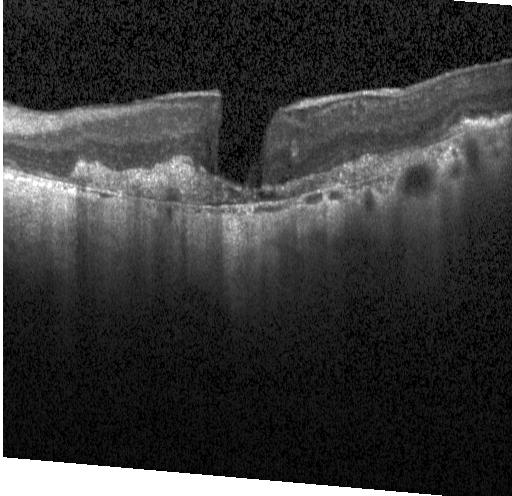 Spectral-domain OCT. Acquired on a Heidelberg Spectralis. Optical coherence tomography scan. Macular scan.
Finding: a choroidal neovascular membrane.